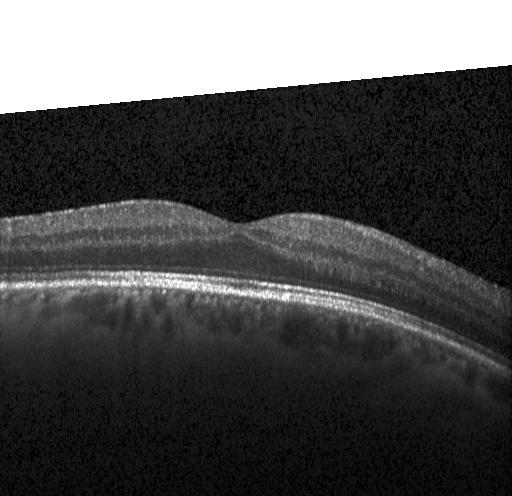 Spectral-domain OCT. OCT B-scan. Instrument: Heidelberg Spectralis — This B-scan demonstrates no CNV, DME, or drusen.